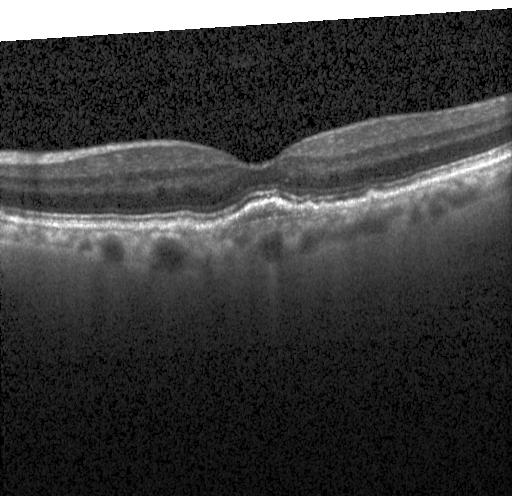
OCT line scan. Instrument: Heidelberg Spectralis. Horizontal scan through the fovea
Finding: a choroidal neovascular membrane.